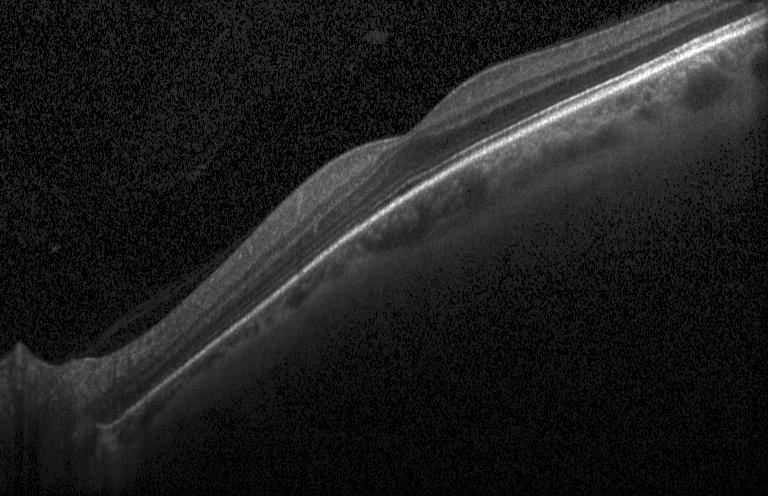
Retinal OCT B-scan. Dx: no CNV, DME, or drusen.